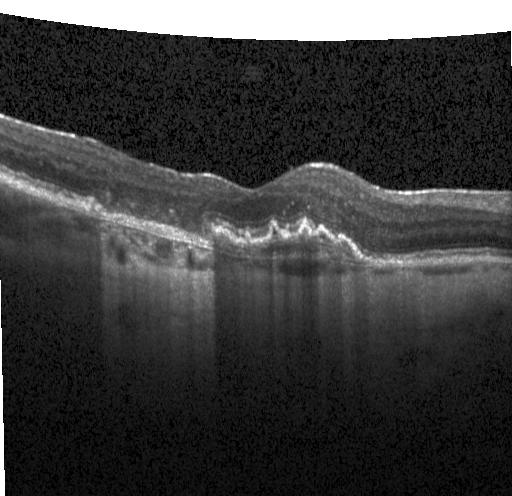 Finding: a choroidal neovascular membrane.